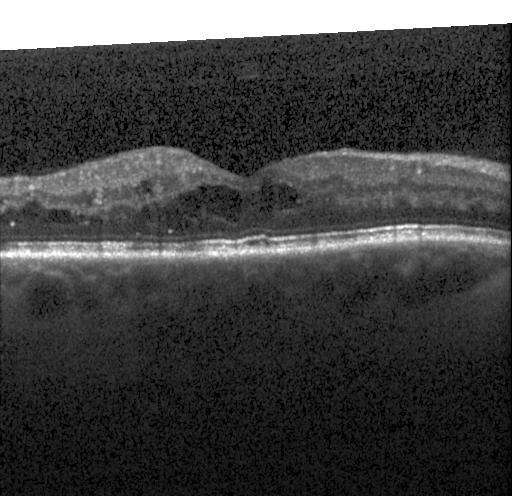
OCT scan showing diabetic macular edema.